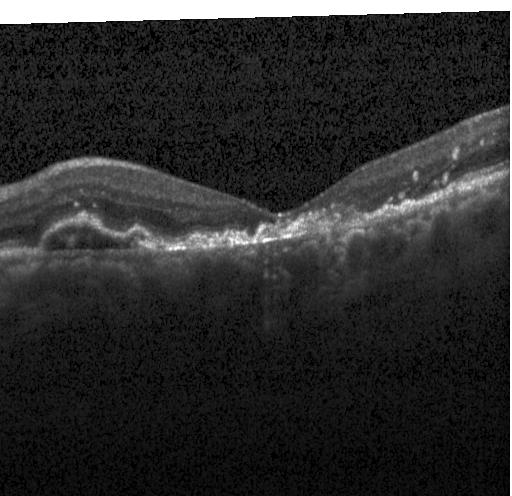

Dx: CNV.